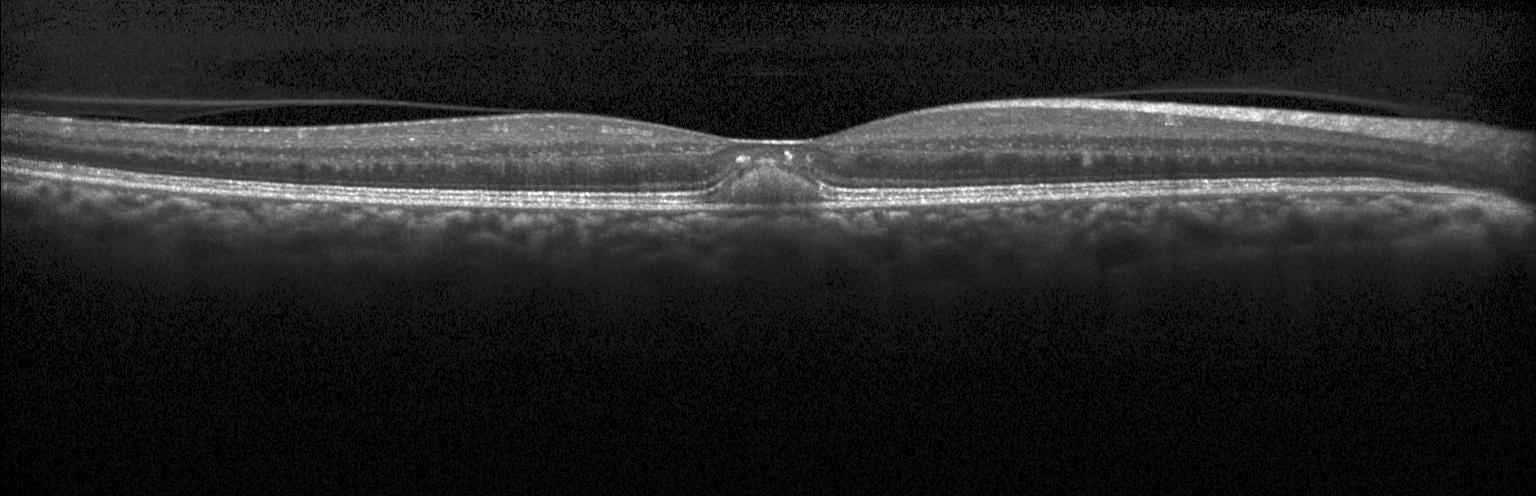
OCT finding: choroidal neovascularization.